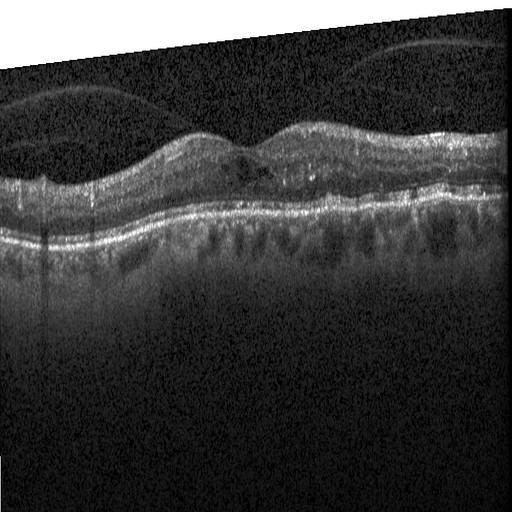 OCT line scan — Impression: diabetic macular edema.